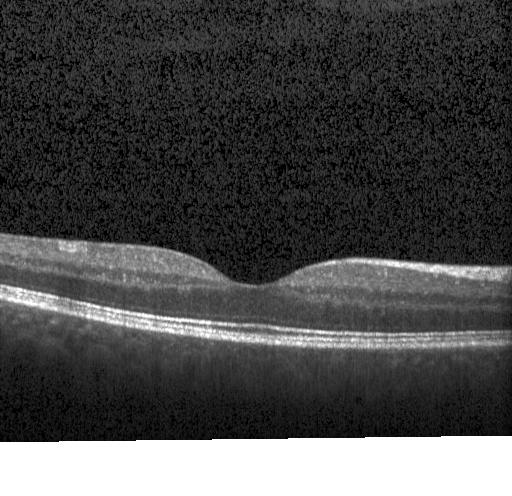 Impression: no evidence of choroidal neovascularization, diabetic macular edema, or drusen.